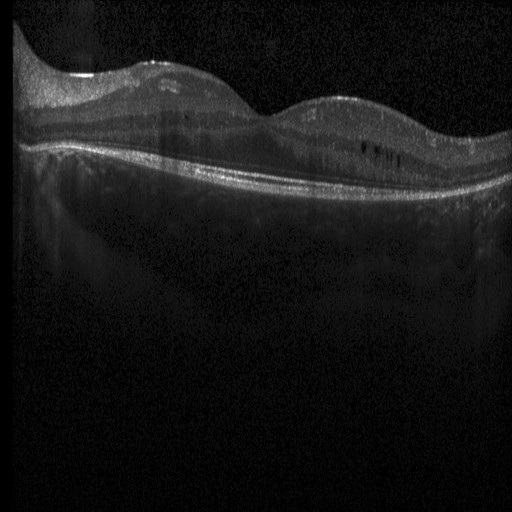 Heidelberg Spectralis OCT system · OCT B-scan.
Diagnosis: diabetic macular edema.